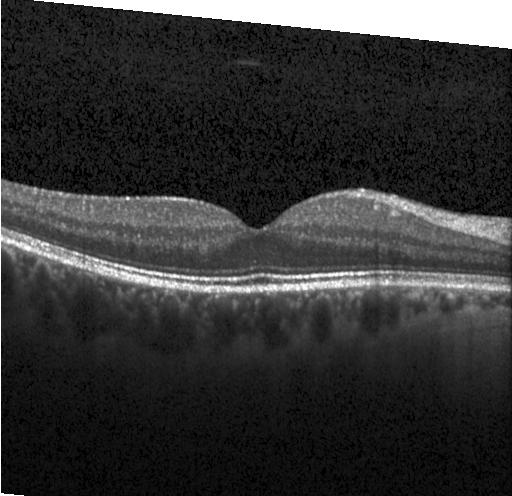

SD-OCT; through the macula; retinal OCT cross-section
OCT finding: no choroidal neovascularization, no diabetic macular edema, and no drusen.